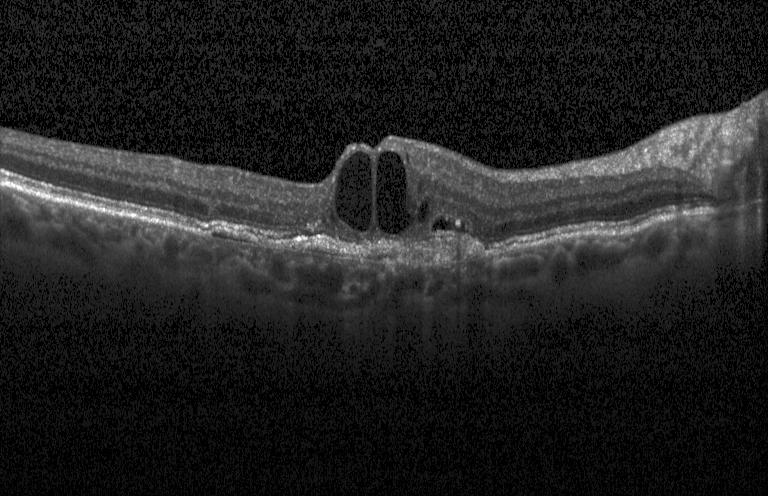 OCT B-scan; Heidelberg Spectralis OCT system; SD-OCT; fovea-centered
Assessment: a choroidal neovascular membrane.